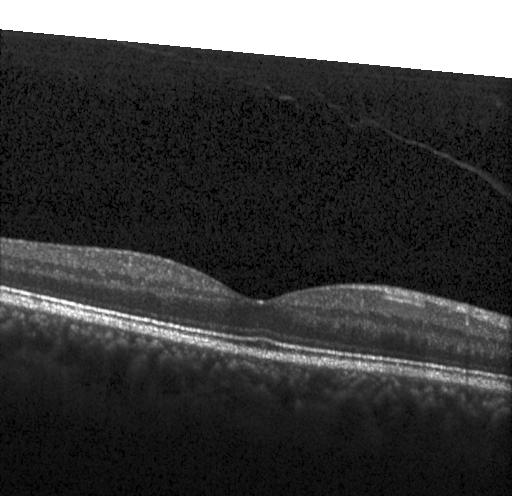

Impression: neither choroidal neovascularization, diabetic macular edema, nor drusen.